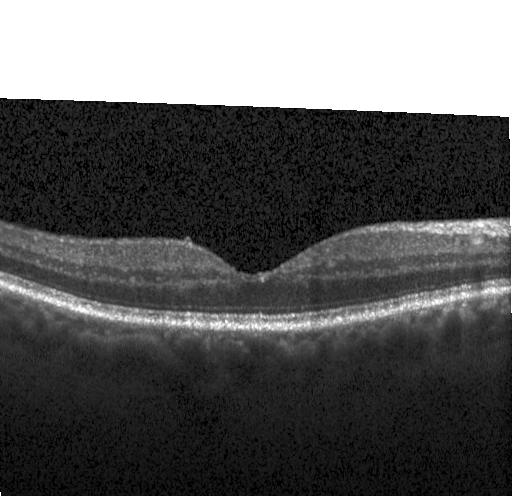

Spectral-domain optical coherence tomography, OCT line scan, through the macula, acquired on a Heidelberg Spectralis. Impression: neither choroidal neovascularization, diabetic macular edema, nor drusen.